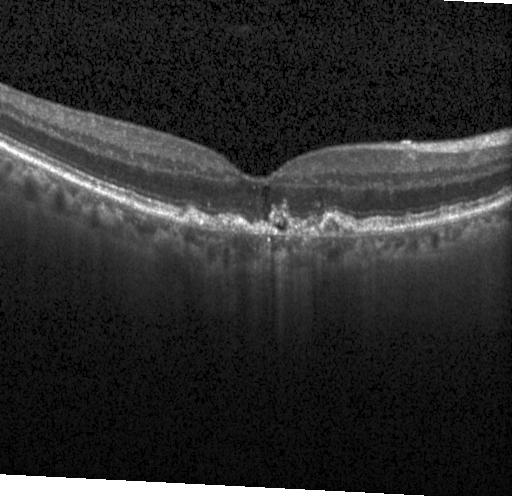
Spectral-domain OCT, centered on the fovea, retinal OCT B-scan, instrument: Heidelberg Spectralis — Diagnosis: a choroidal neovascular membrane.